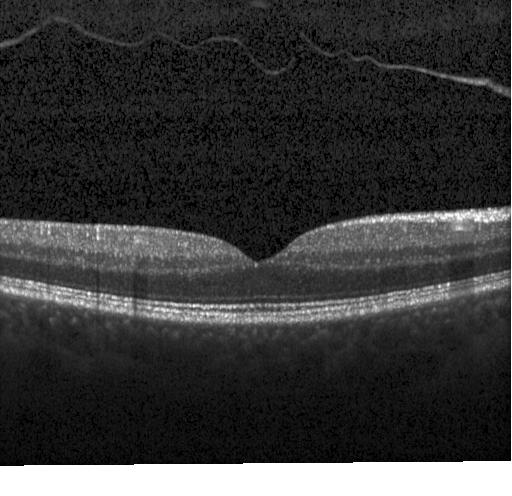 OCT scan showing neither choroidal neovascularization, diabetic macular edema, nor drusen.